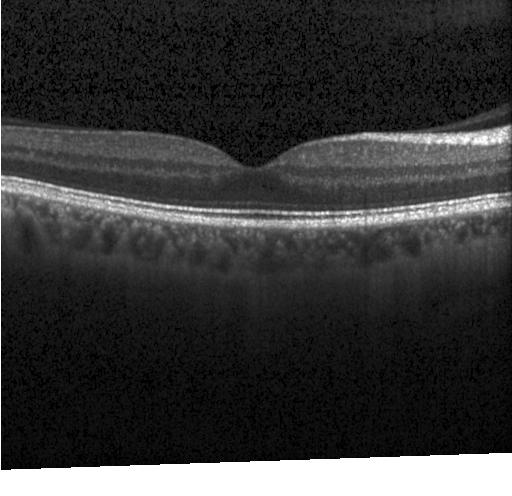
Impression: neither choroidal neovascularization, diabetic macular edema, nor drusen.